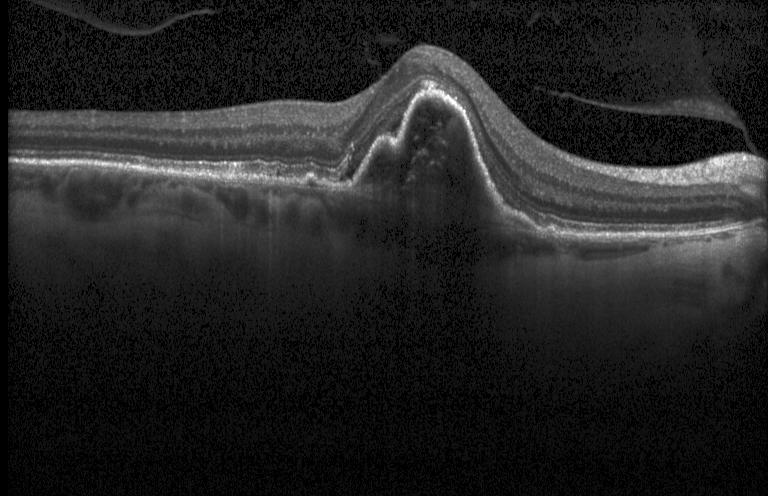

Spectral-domain OCT, instrument: Heidelberg Spectralis, OCT B-scan, fovea-centered. A choroidal neovascular membrane.